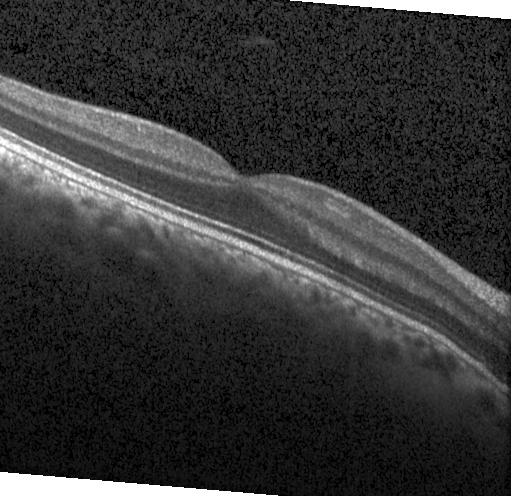
Macular OCT: no choroidal neovascularization, no diabetic macular edema, and no drusen.